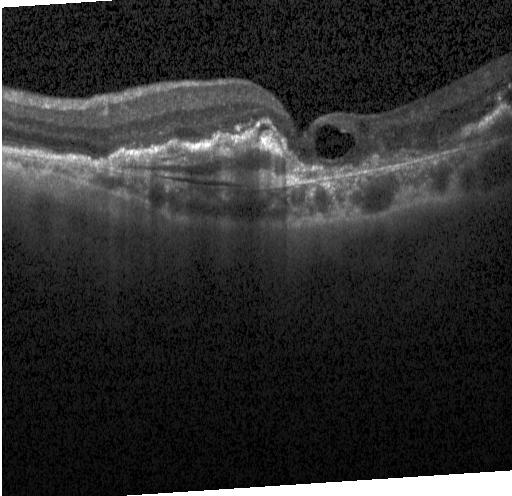 OCT B-scan showing CNV.